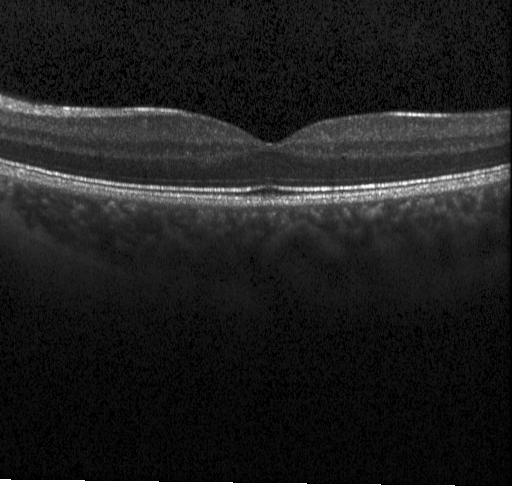

Spectral-domain optical coherence tomography · optical coherence tomography B-scan · horizontal scan through the fovea · Heidelberg Spectralis — Assessment: no CNV, DME, or drusen.